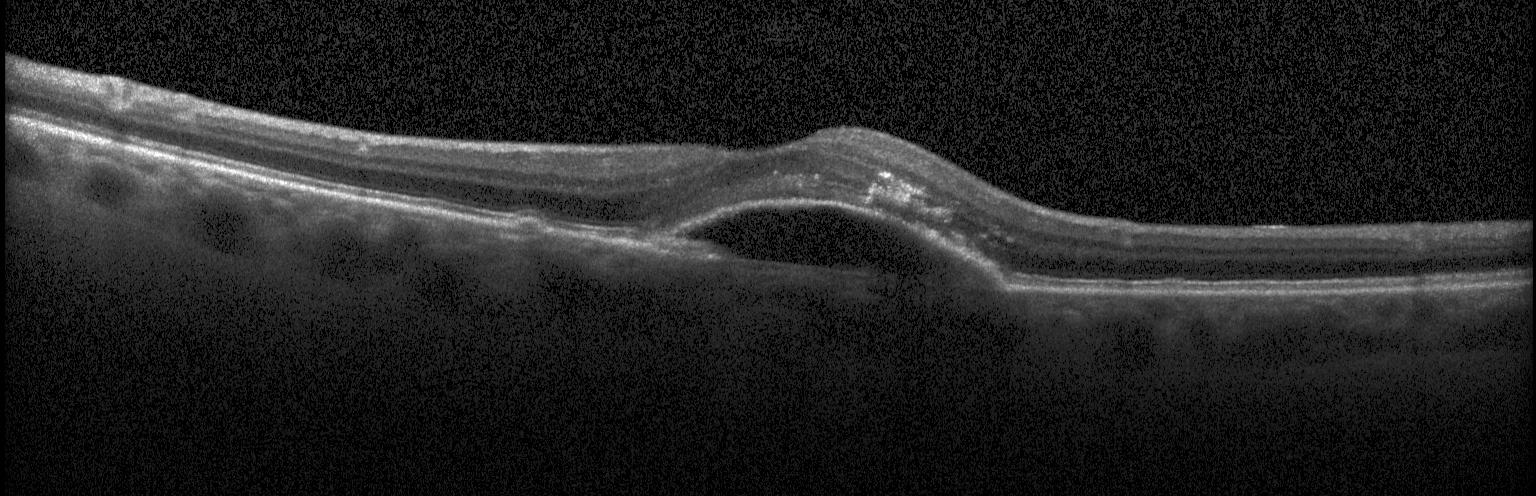

Heidelberg Spectralis; spectral-domain OCT; OCT line scan
OCT finding: choroidal neovascularization (CNV).